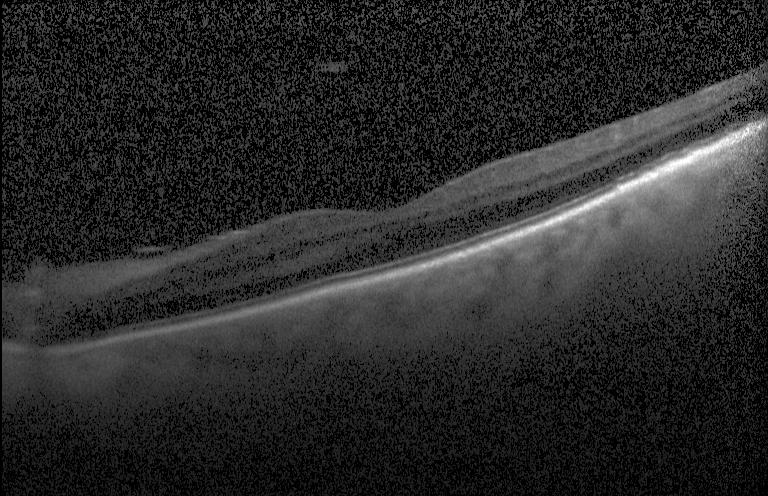 Spectral-domain OCT B-scan: no choroidal neovascularization, no diabetic macular edema, and no drusen.